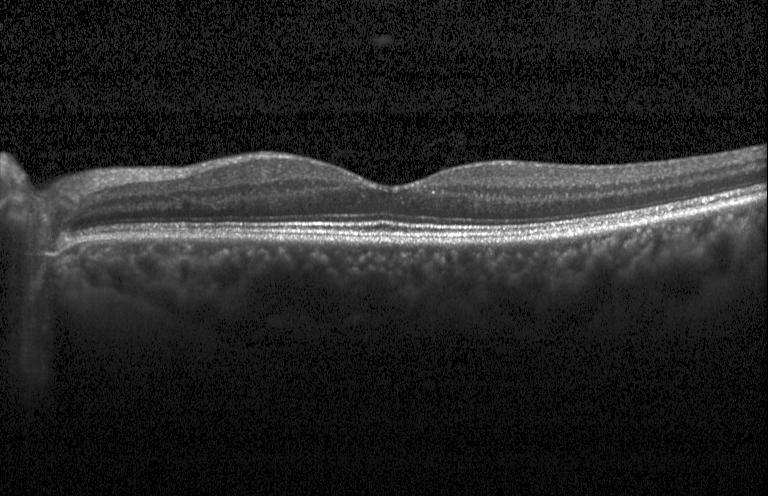
Optical coherence tomography scan · fovea-centered.
Impression: no CNV, no DME, and no drusen.